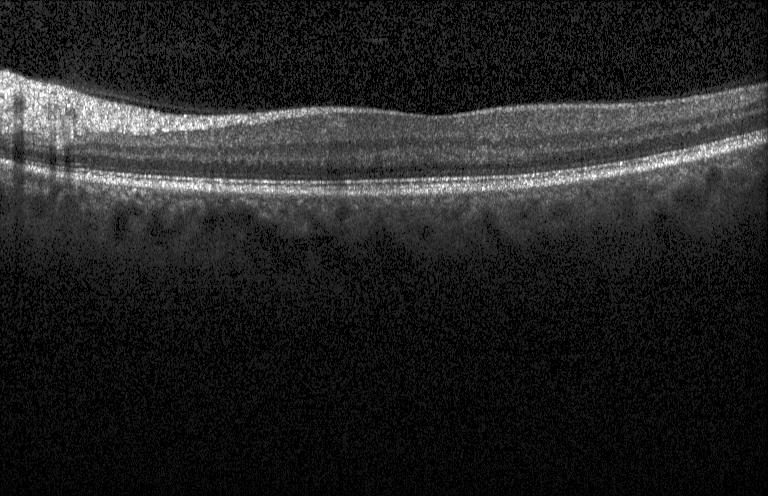

Optical coherence tomography scan · SD-OCT · instrument: Heidelberg Spectralis — This B-scan demonstrates no choroidal neovascularization, diabetic macular edema, or drusen.